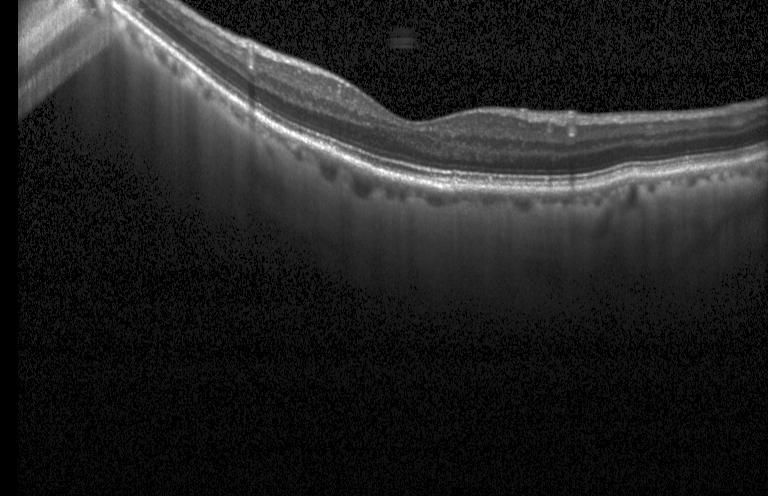
Macular scan, acquired on a Heidelberg Spectralis, optical coherence tomography scan. Impression: no choroidal neovascularization, no diabetic macular edema, and no drusen.